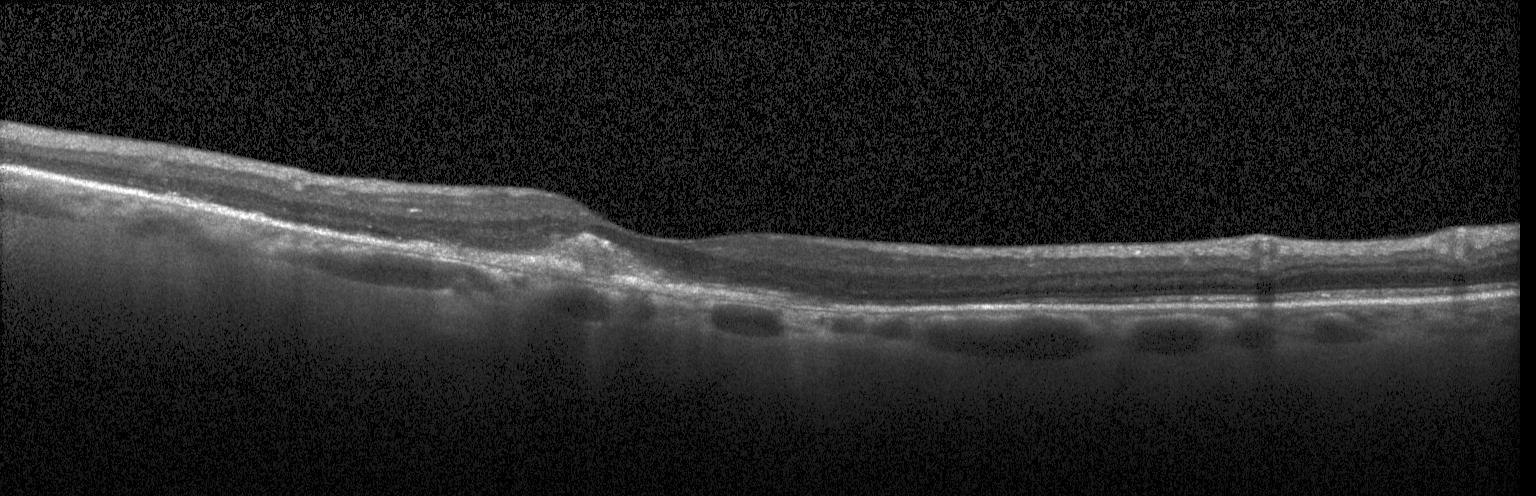 Instrument: Heidelberg Spectralis; macular scan; OCT line scan. Impression: choroidal neovascularization.